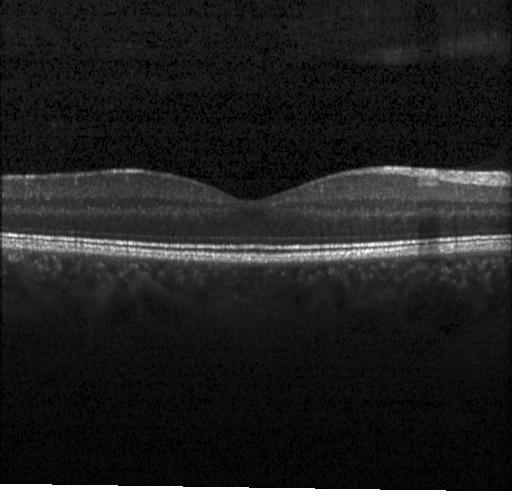
Optical coherence tomography B-scan. No evidence of choroidal neovascularization, diabetic macular edema, or drusen.